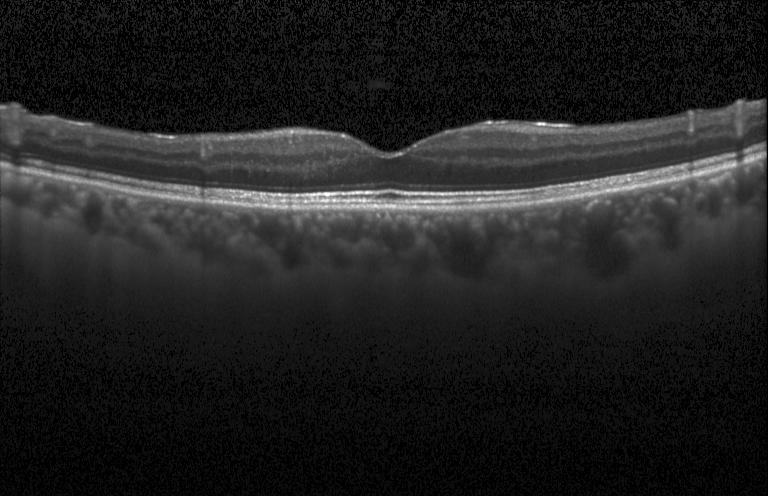
OCT B-scan showing no evidence of CNV, DME, or drusen.